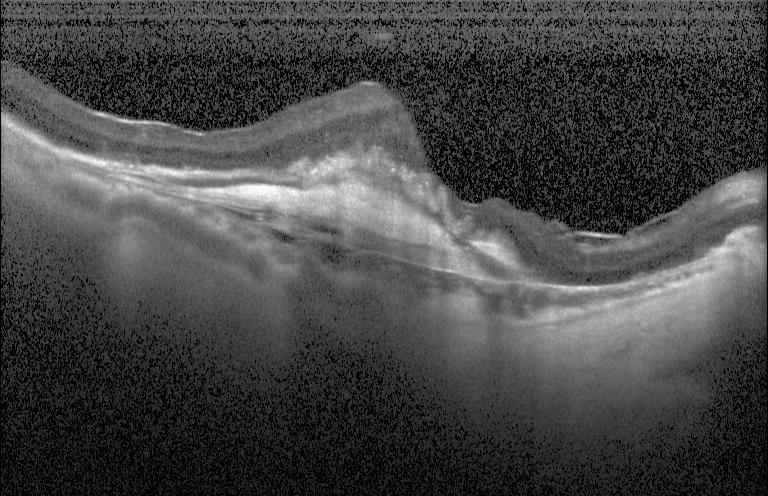
SD-OCT, fovea-centered, retinal OCT cross-section — Dx: CNV.